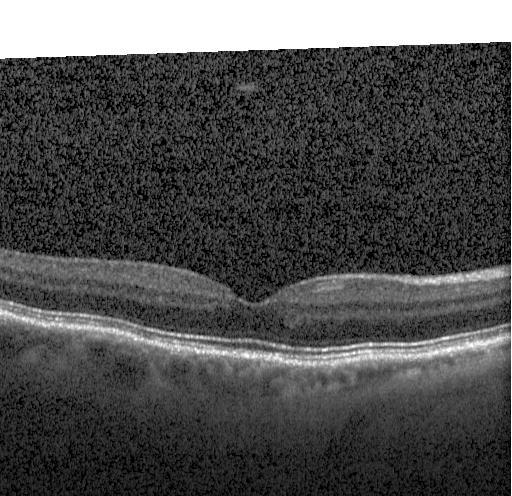 Impression: no choroidal neovascularization, no diabetic macular edema, and no drusen.